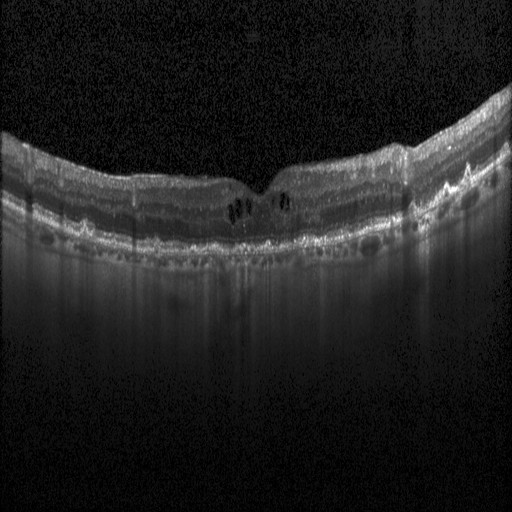 OCT finding: diabetic macular edema (DME).